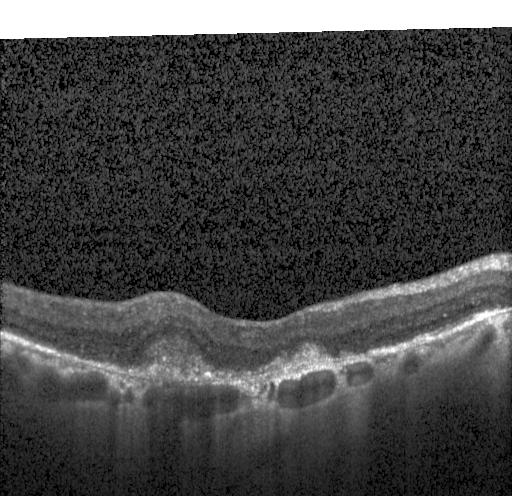

Optical coherence tomography B-scan, spectral-domain optical coherence tomography, Heidelberg Spectralis. Impression: choroidal neovascularization (CNV).